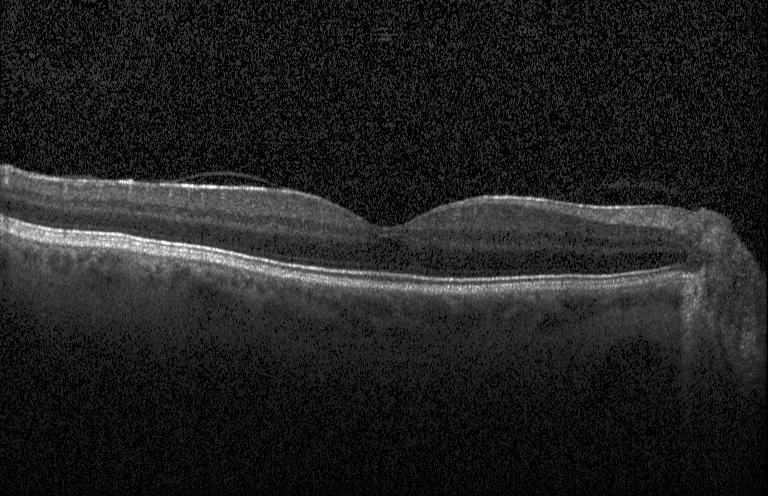
Retinal OCT B-scan
No CNV, DME, or drusen.